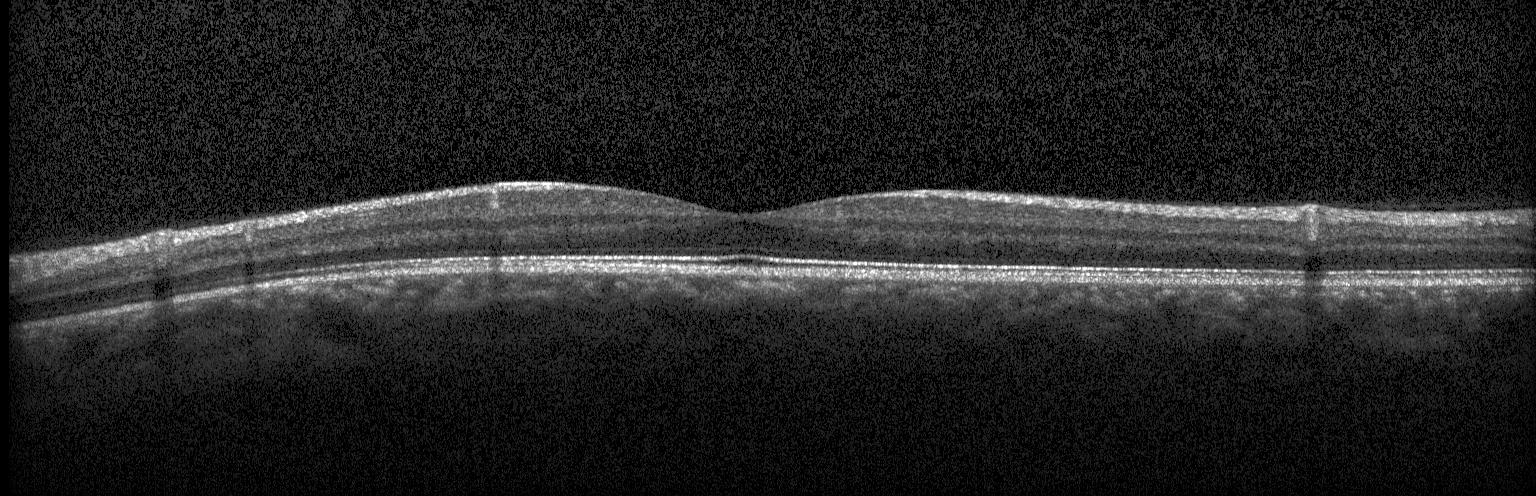

Optical coherence tomography scan — Diagnosis: neither choroidal neovascularization, diabetic macular edema, nor drusen.